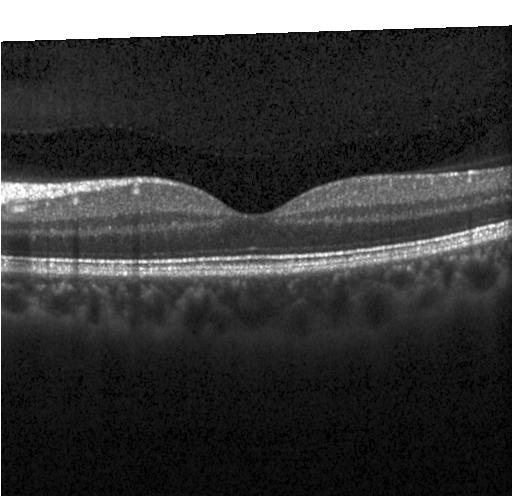 Impression: no evidence of choroidal neovascularization, diabetic macular edema, or drusen.